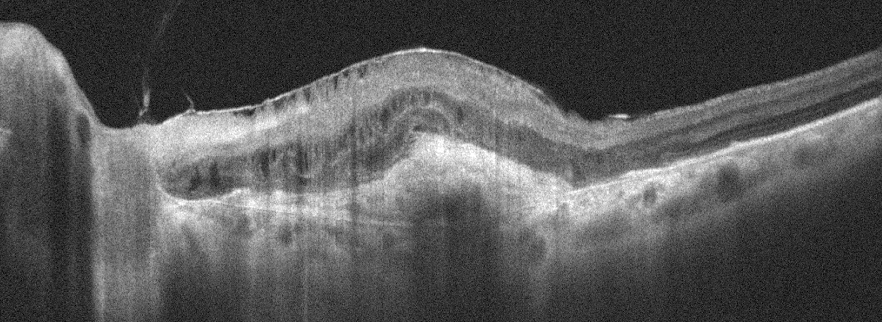
Retinal OCT cross-section showing age-related macular degeneration.